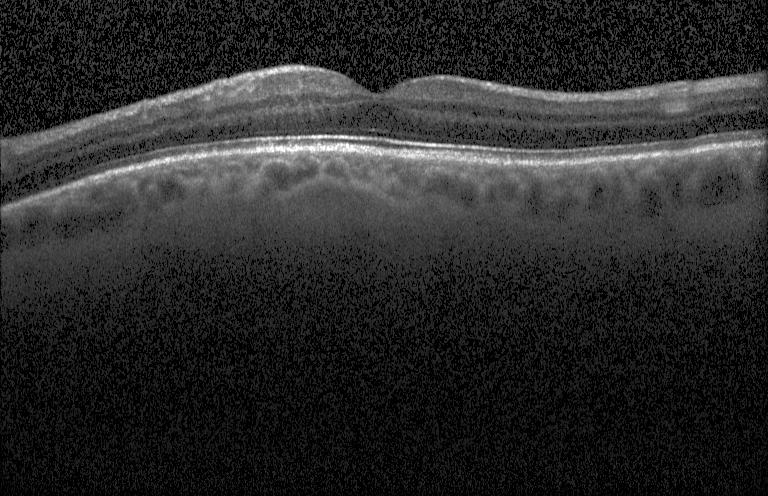 Assessment: no evidence of choroidal neovascularization, diabetic macular edema, or drusen.